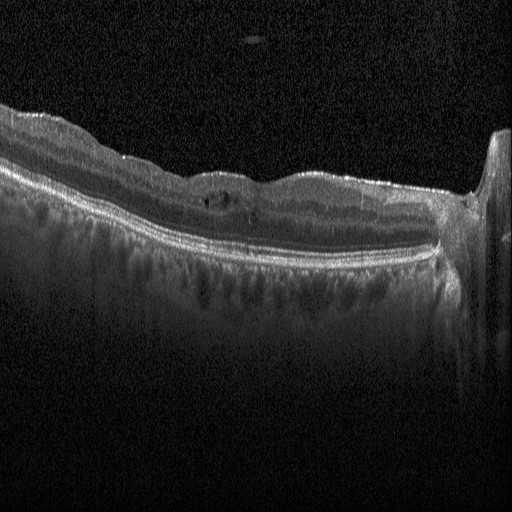
Diagnosis: diabetic macular edema (DME).